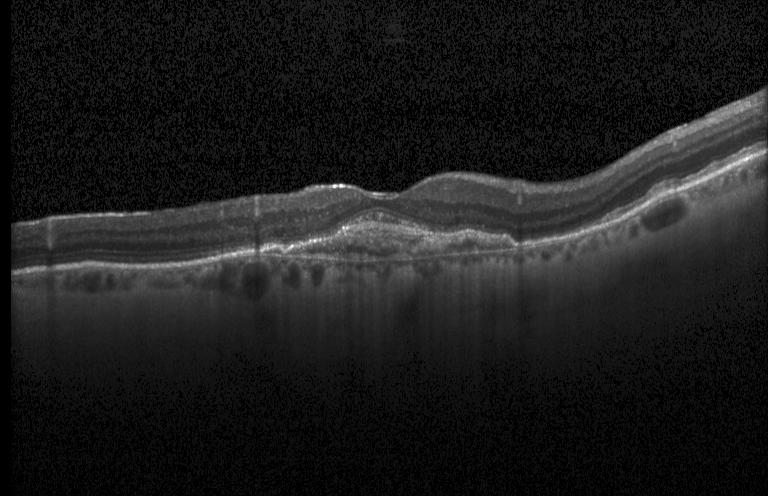 Retinal OCT cross-section showing CNV.